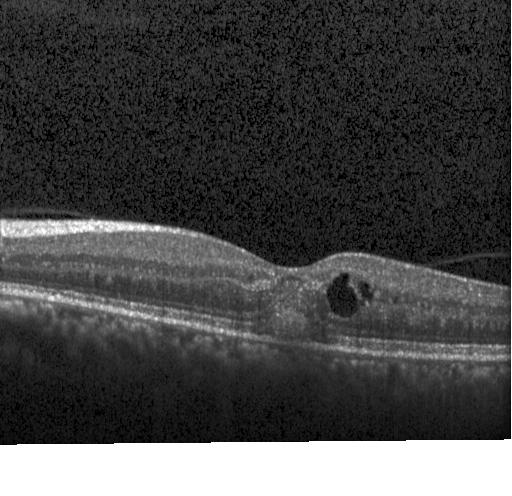

Retinal OCT cross-section — Assessment: a choroidal neovascular membrane.